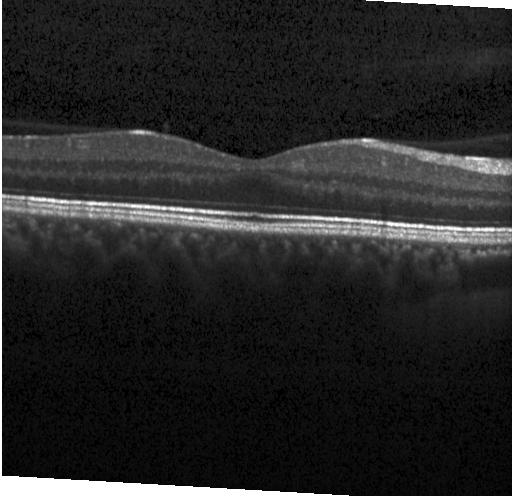

Macular scan, OCT line scan.
Impression: no evidence of choroidal neovascularization, diabetic macular edema, or drusen.